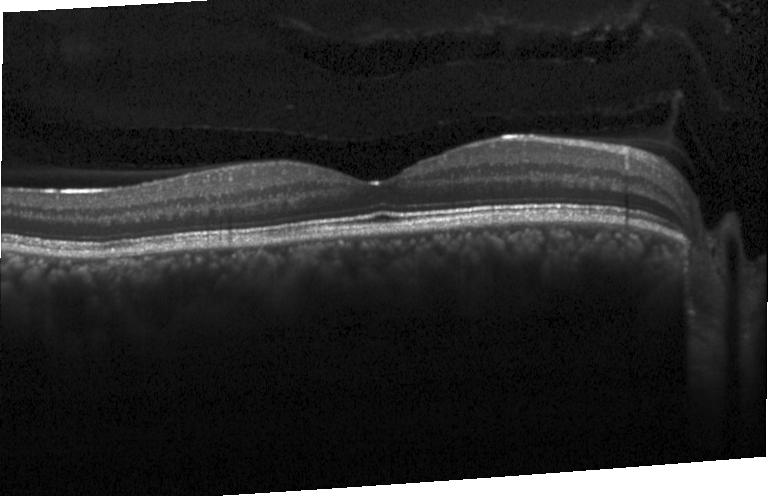

Optical coherence tomography scan.
OCT finding: no choroidal neovascularization, diabetic macular edema, or drusen.